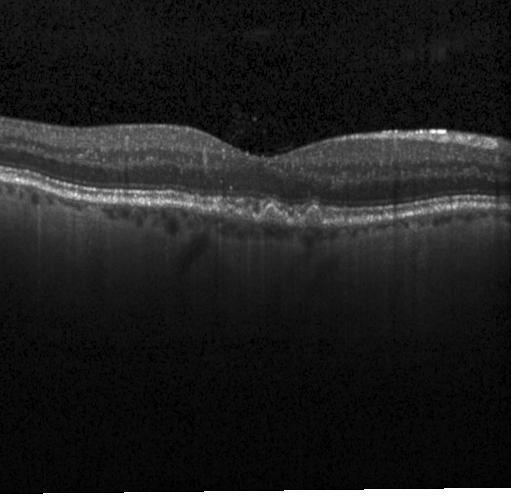
Macular OCT: multiple drusen.